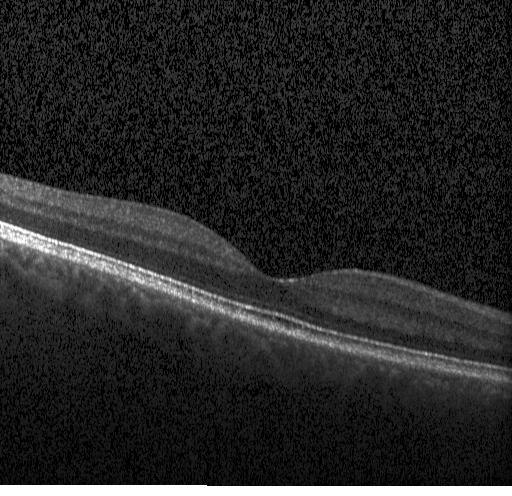

Dx: neither choroidal neovascularization, diabetic macular edema, nor drusen.